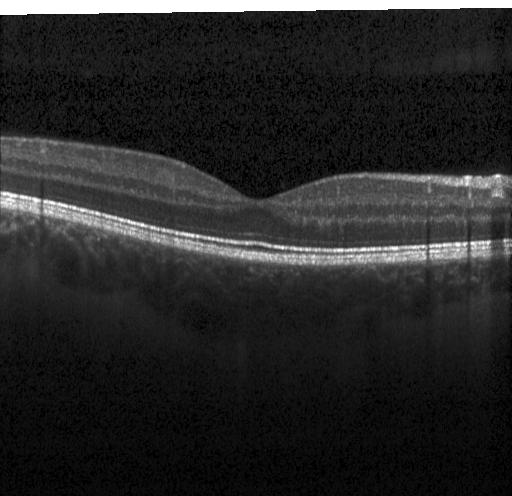 Retinal OCT cross-section.
Finding: no evidence of choroidal neovascularization, diabetic macular edema, or drusen.